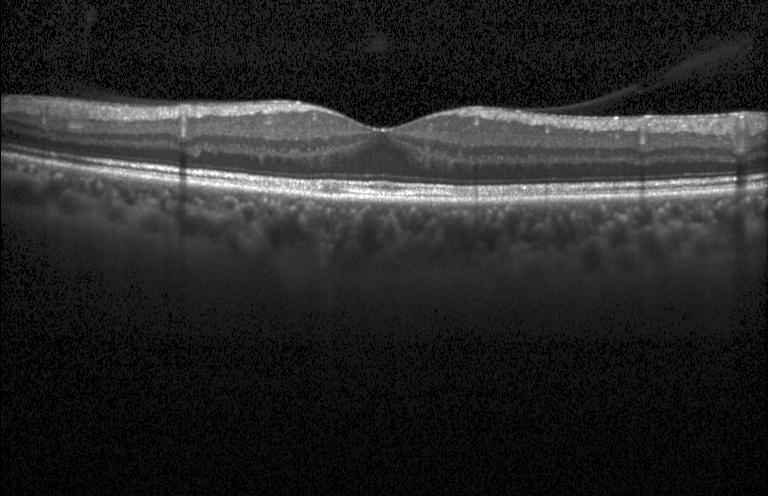 OCT scan showing no choroidal neovascularization, diabetic macular edema, or drusen.